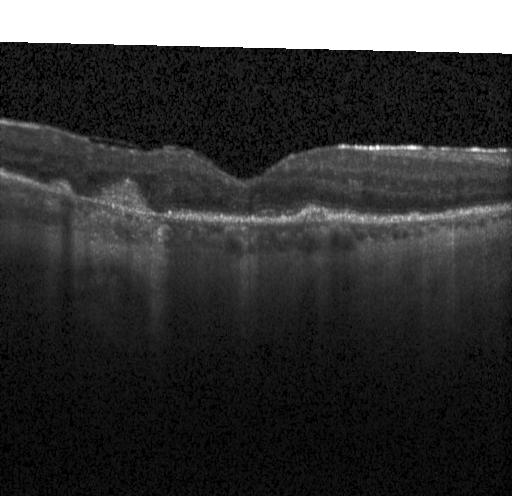

Heidelberg Spectralis; spectral-domain optical coherence tomography; through the macula; OCT line scan — Assessment: a choroidal neovascular membrane.